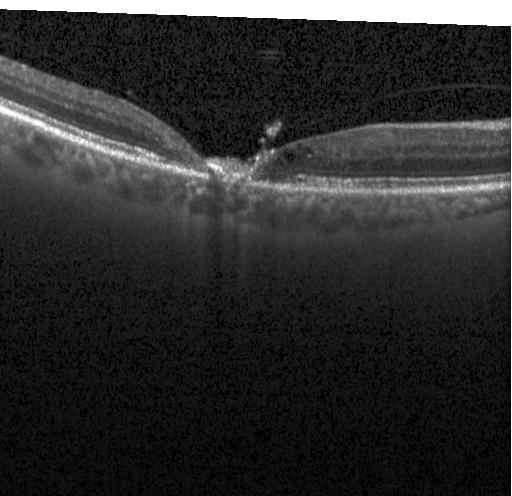
Diagnosis: a choroidal neovascular membrane.